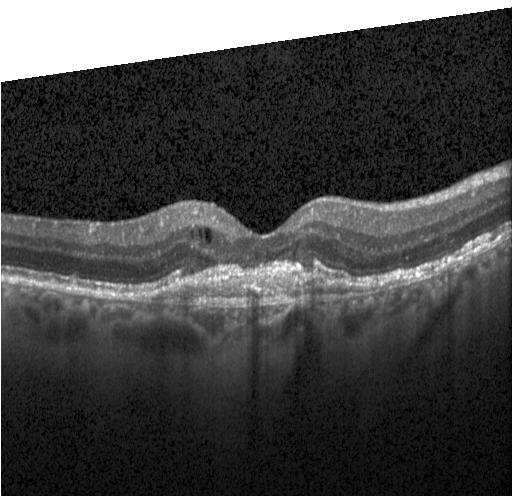
This B-scan demonstrates CNV.